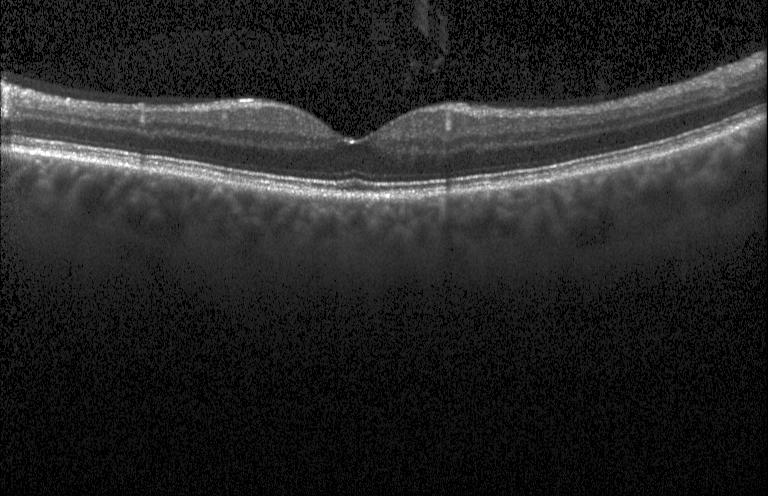

Spectral-domain optical coherence tomography. Heidelberg Spectralis. Retinal OCT B-scan — Assessment: no choroidal neovascularization, no diabetic macular edema, and no drusen.